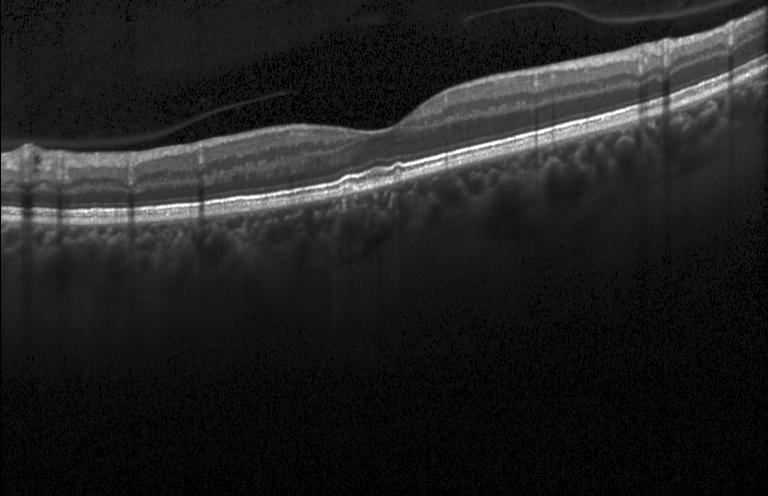 Optical coherence tomography B-scan
Impression: sub-RPE drusenoid deposits.